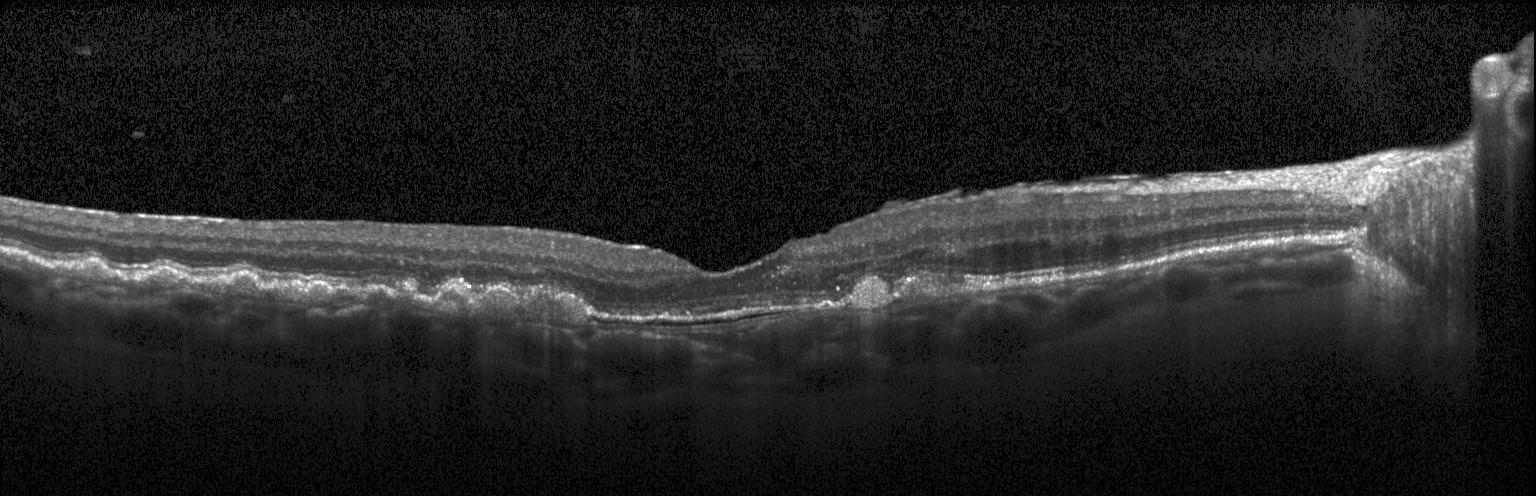

Optical coherence tomography scan; Heidelberg Spectralis OCT system; SD-OCT.
Finding: choroidal neovascularization (CNV).